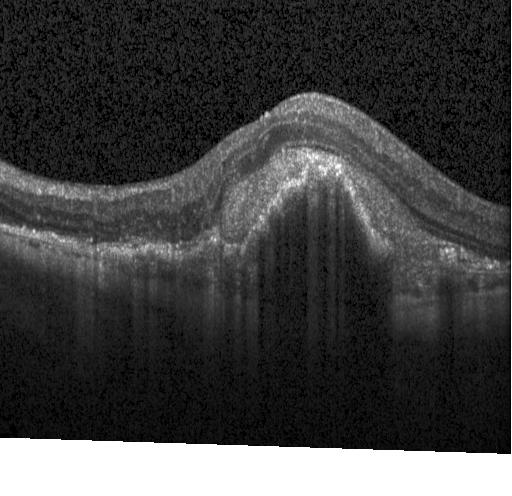 Optical coherence tomography scan — The scan shows CNV.